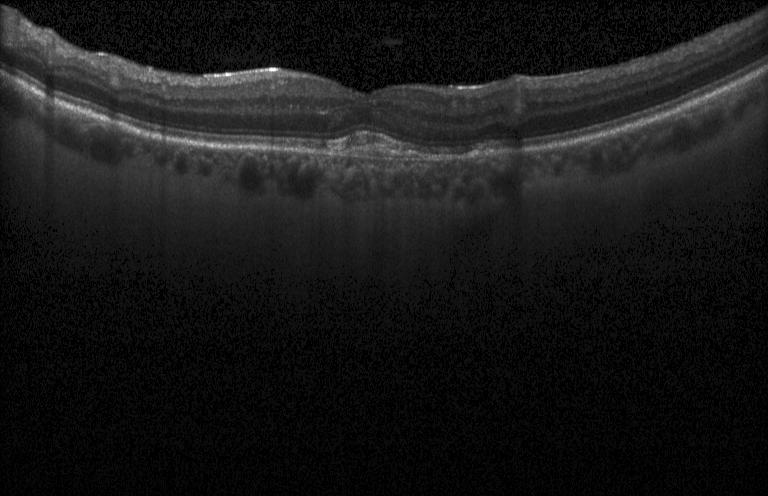
Spectral-domain optical coherence tomography, Heidelberg Spectralis, optical coherence tomography scan, fovea-centered
OCT finding: a choroidal neovascular membrane.